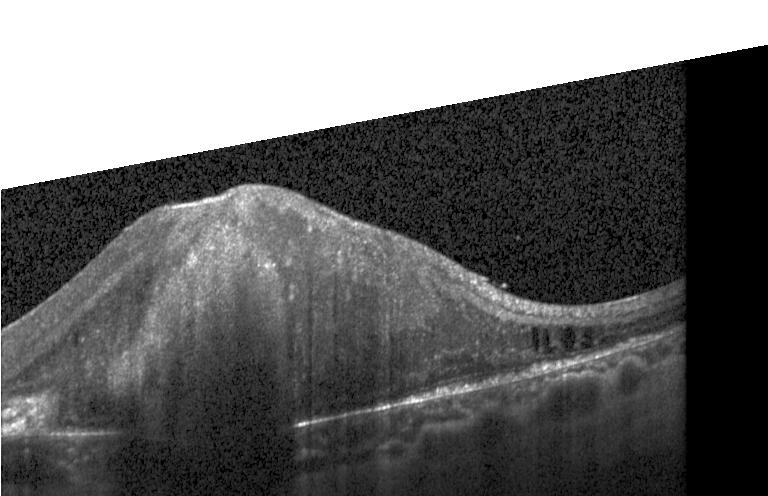
Heidelberg Spectralis OCT system; spectral-domain OCT; retinal OCT cross-section; through the macula. Assessment: a choroidal neovascular membrane.